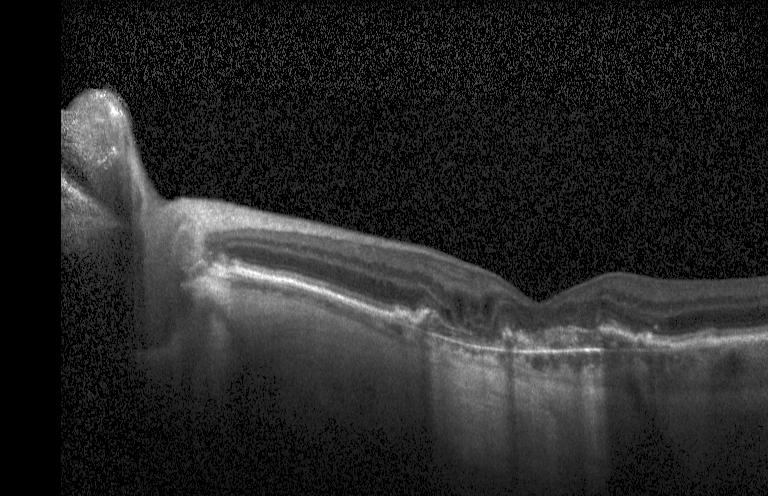 Impression: CNV.